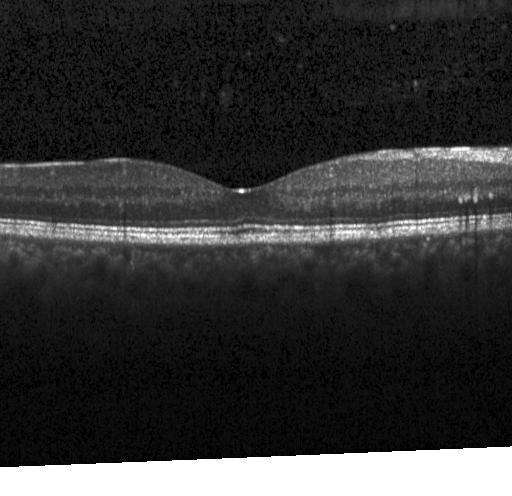

No CNV, DME, or drusen.